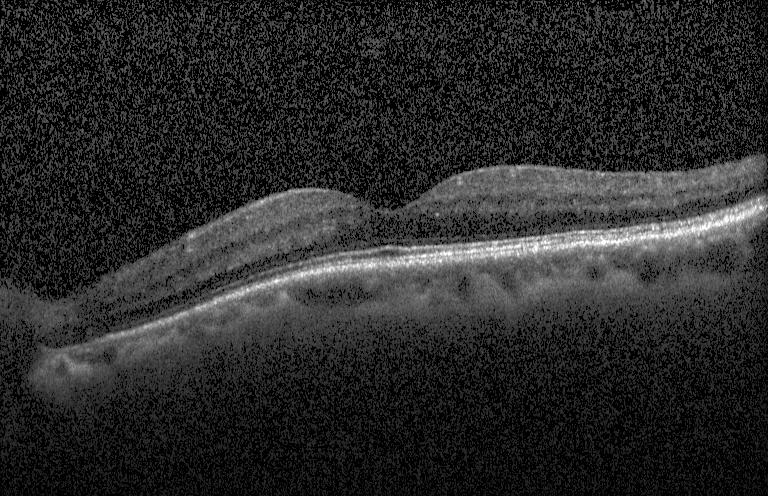
SD-OCT, acquired on a Heidelberg Spectralis, optical coherence tomography scan, macular scan — This B-scan demonstrates no evidence of choroidal neovascularization, diabetic macular edema, or drusen.